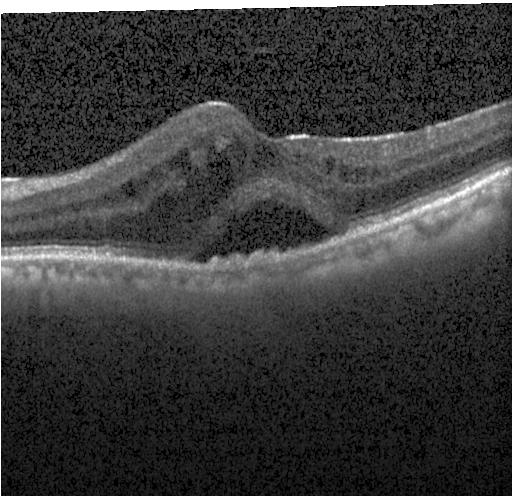
OCT line scan, spectral-domain OCT
Finding: DME.